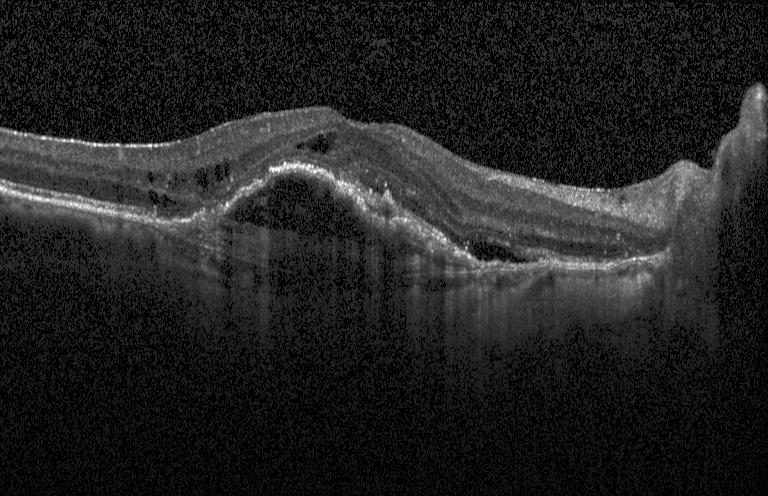
Retinal OCT B-scan — Dx: choroidal neovascularization.